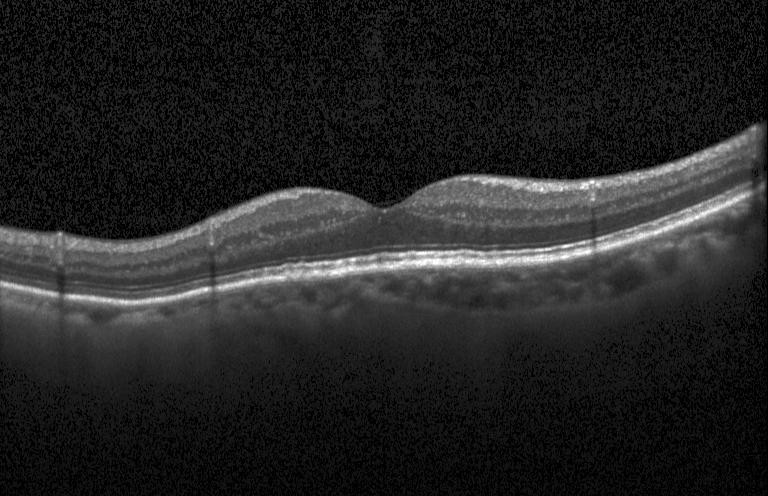 OCT finding: no CNV, no DME, and no drusen.